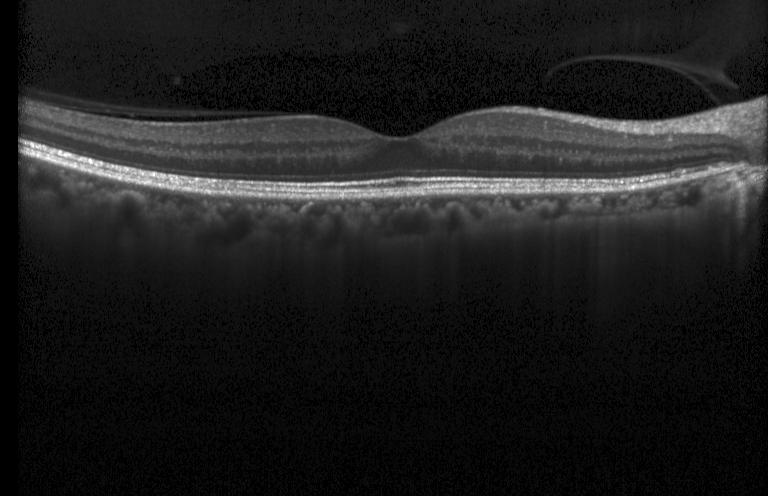

Assessment: no choroidal neovascularization, diabetic macular edema, or drusen.